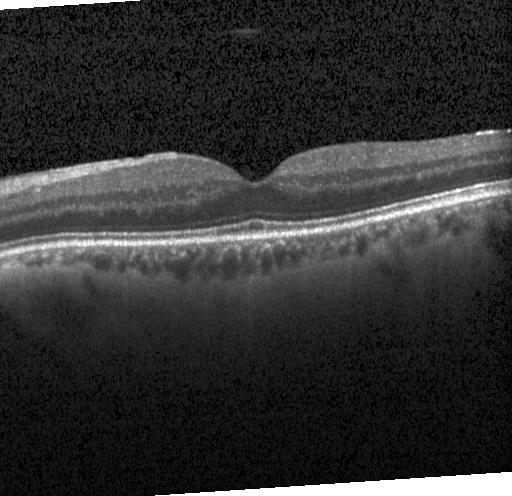
Dx: no evidence of CNV, DME, or drusen.